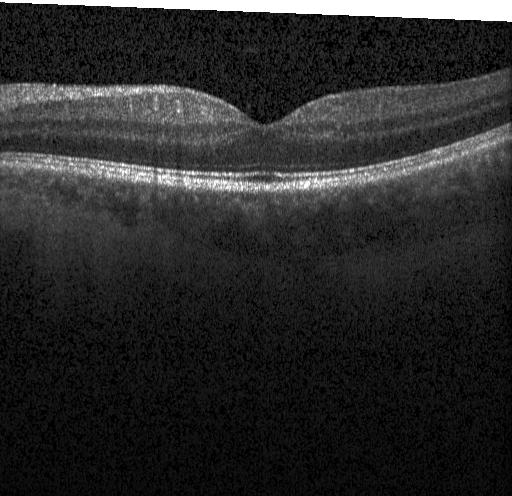

OCT B-scan showing no CNV, no DME, and no drusen.